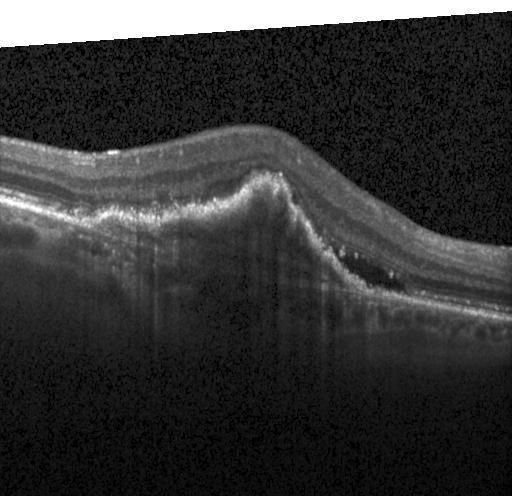
OCT line scan; SD-OCT — Finding: choroidal neovascularization (CNV).